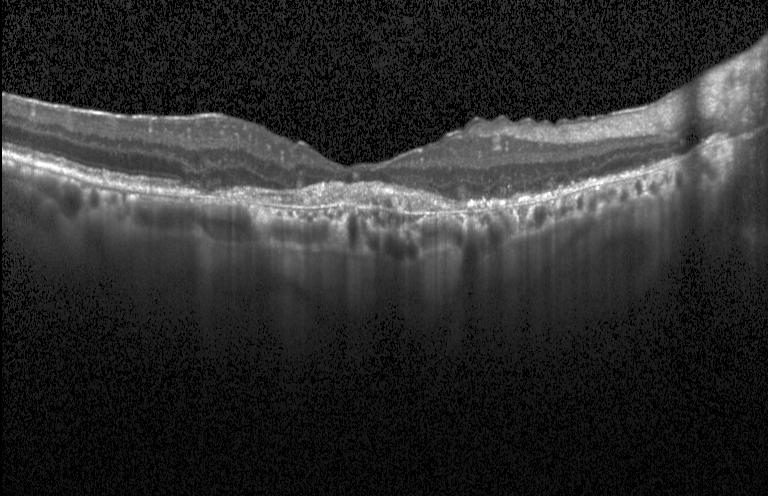

Retinal OCT cross-section; Heidelberg Spectralis. Macular OCT: CNV.